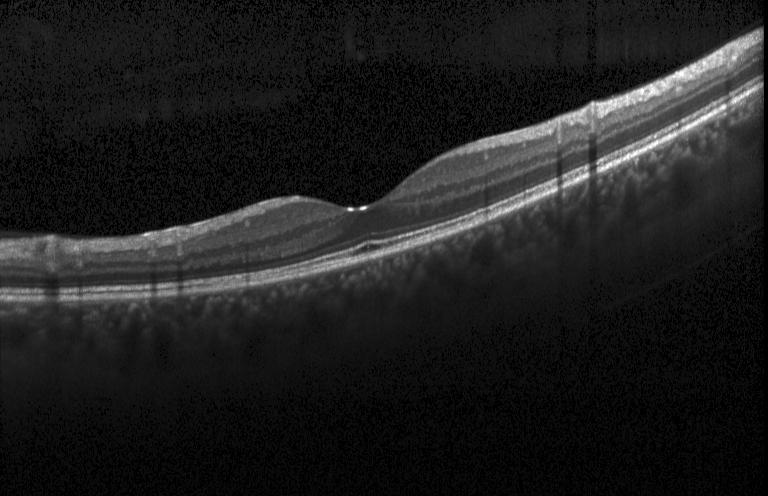

Dx: no CNV, DME, or drusen.